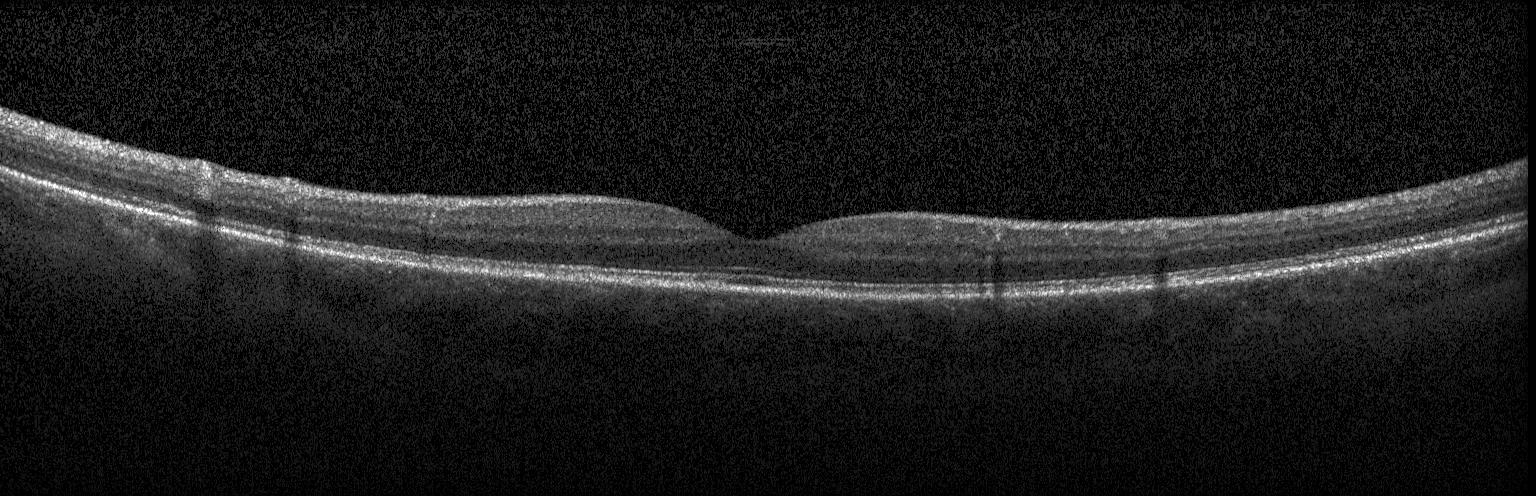 OCT line scan · fovea-centered — Impression: no choroidal neovascularization, diabetic macular edema, or drusen.